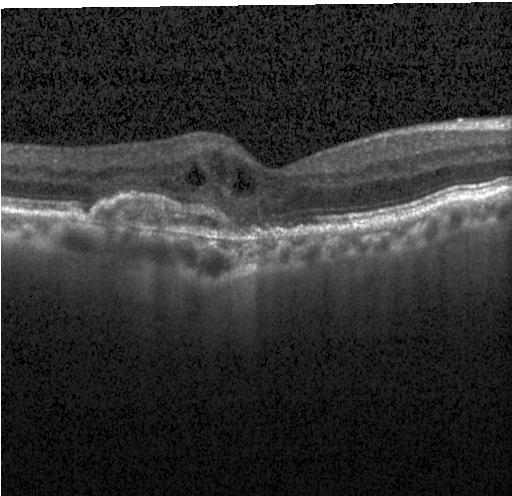 OCT line scan; acquired on a Heidelberg Spectralis; horizontal scan through the fovea; SD-OCT.
Finding: choroidal neovascularization (CNV).